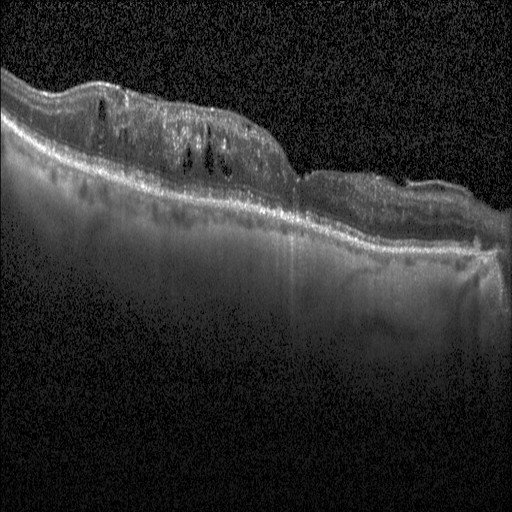 Fovea-centered; OCT B-scan; SD-OCT; instrument: Heidelberg Spectralis — Impression: diabetic macular edema (DME).